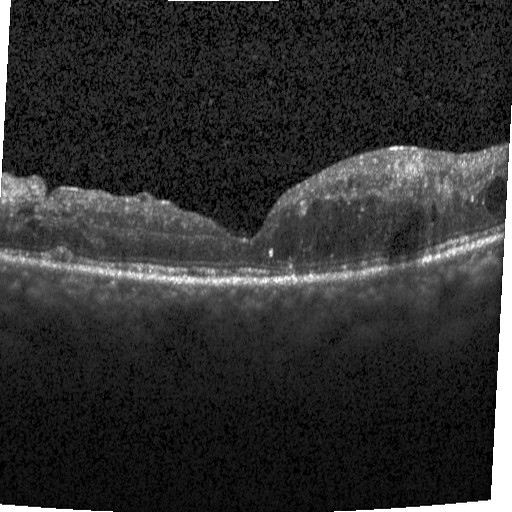 Optical coherence tomography scan.
Finding: diabetic macular edema (DME).